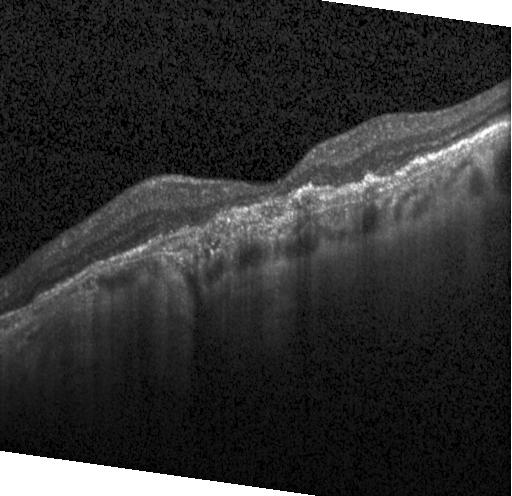
Retinal OCT cross-section showing choroidal neovascularization.